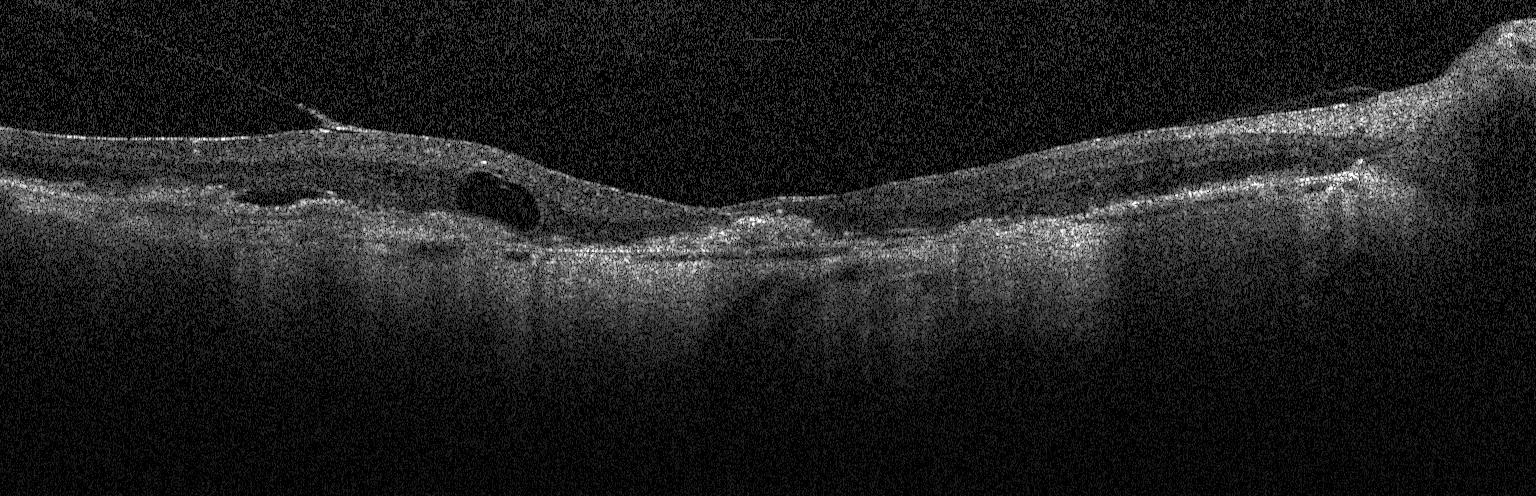

Spectral-domain OCT B-scan: CNV.